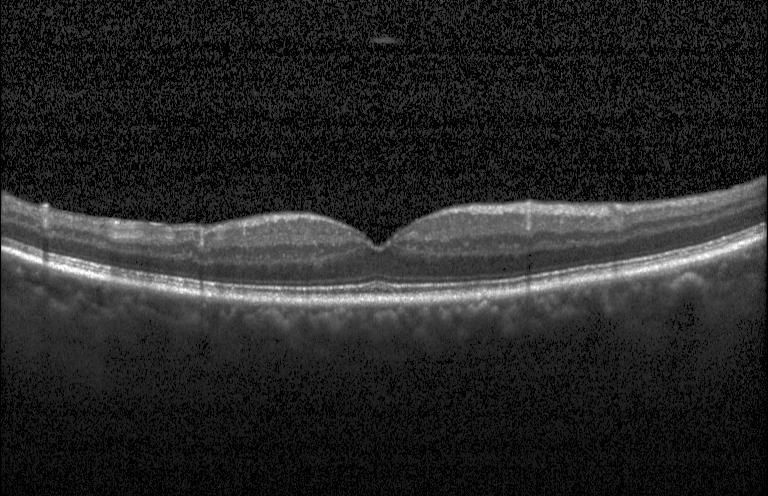 Retinal OCT cross-section · acquired on a Heidelberg Spectralis. Dx: no choroidal neovascularization, diabetic macular edema, or drusen.